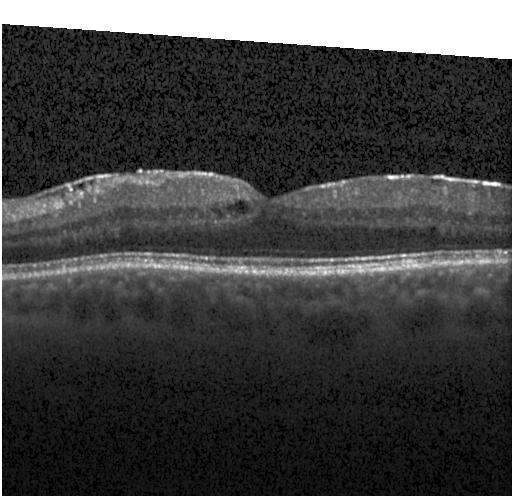 This B-scan demonstrates diabetic macular edema.